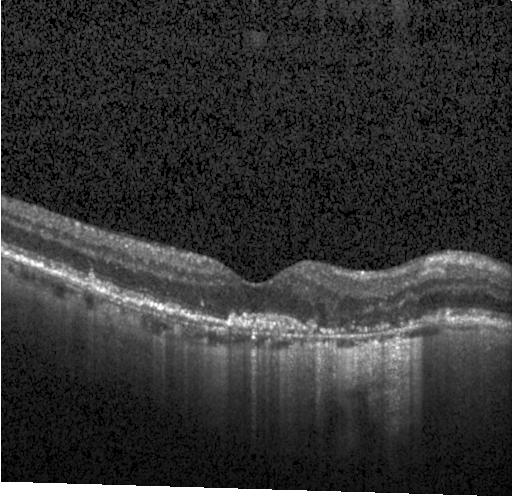

Impression: a choroidal neovascular membrane.